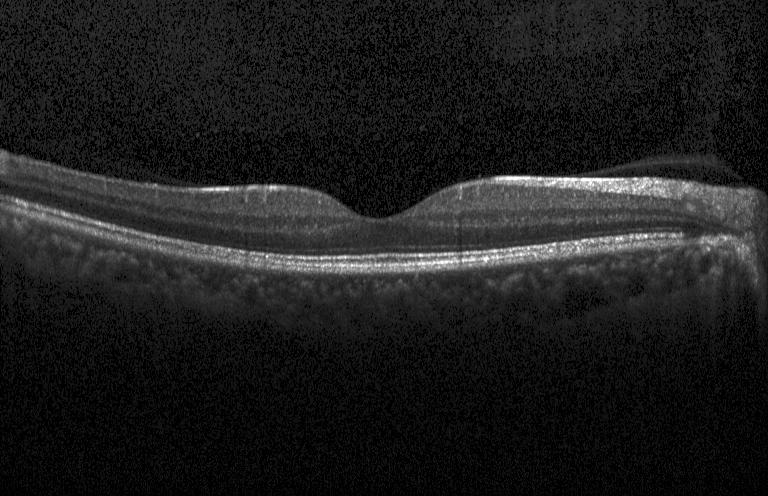
Retinal OCT B-scan
This B-scan demonstrates no CNV, DME, or drusen.